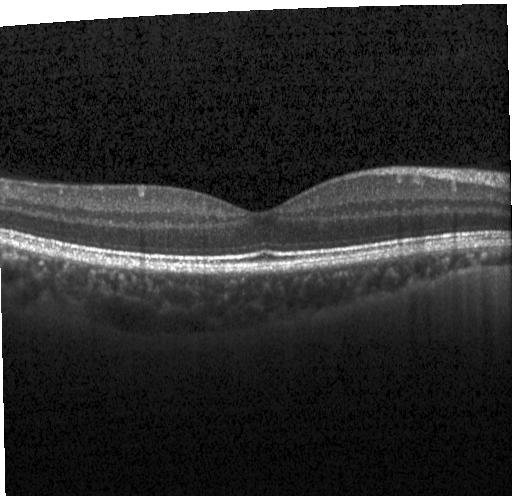

Diagnosis: no evidence of CNV, DME, or drusen.